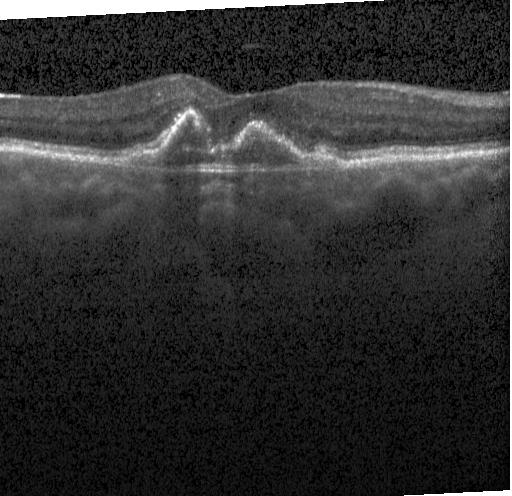 Retinal OCT cross-section, spectral-domain OCT, instrument: Heidelberg Spectralis.
Finding: a choroidal neovascular membrane.